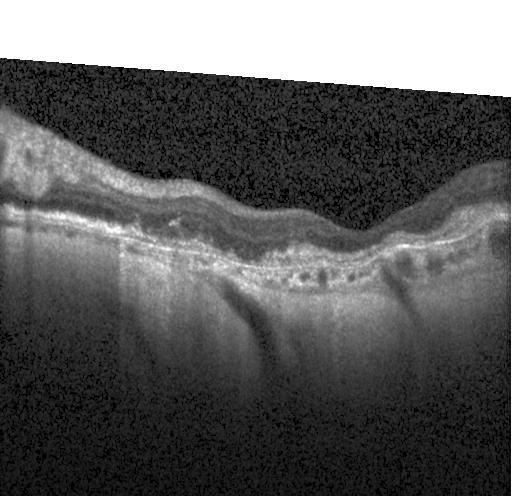 Assessment: a choroidal neovascular membrane.